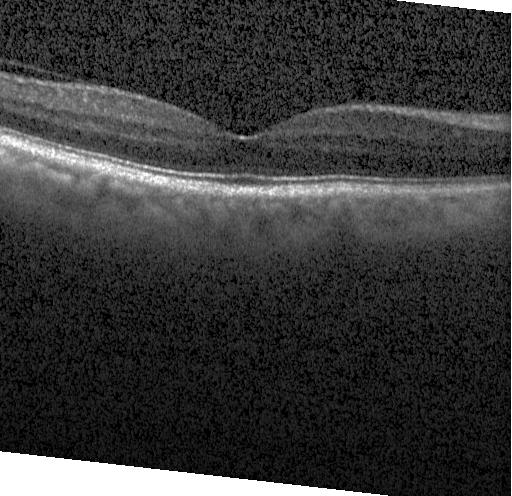 Finding: no choroidal neovascularization, no diabetic macular edema, and no drusen.